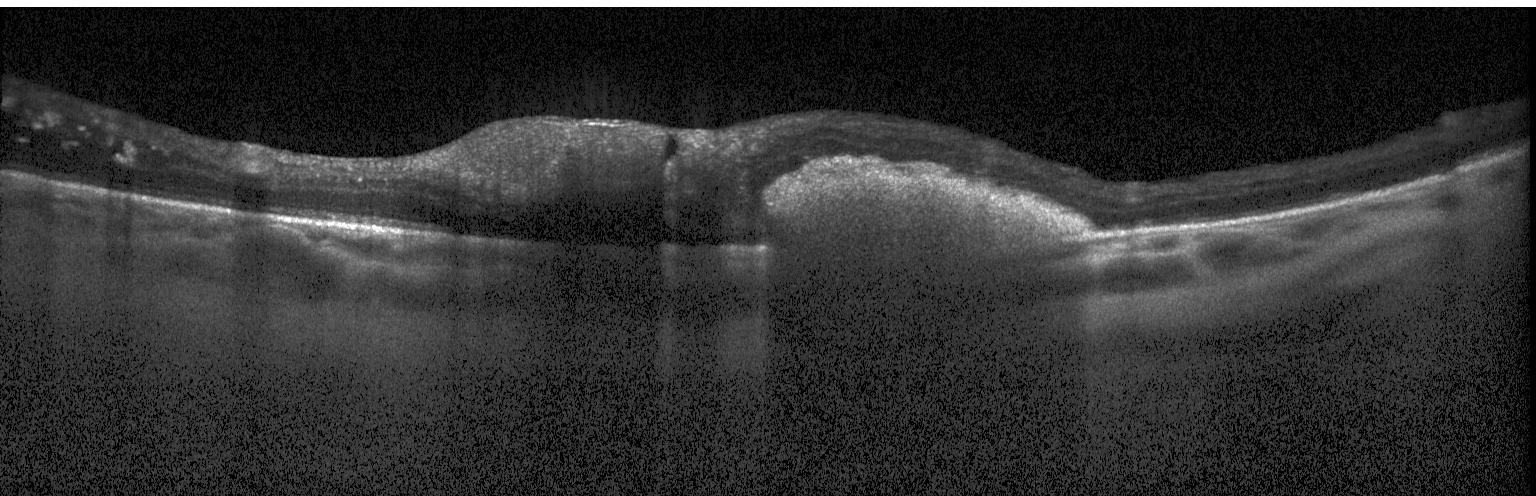
Dx: CNV.